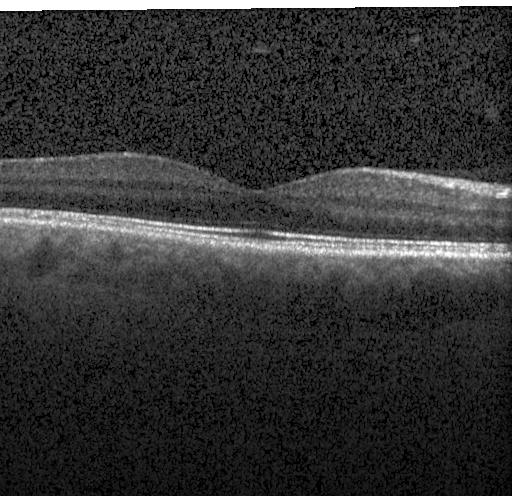

Diagnosis: no evidence of choroidal neovascularization, diabetic macular edema, or drusen.